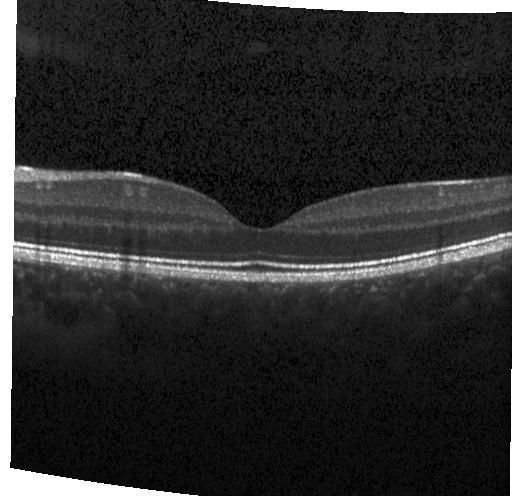

Retinal OCT cross-section · spectral-domain OCT. Finding: no evidence of choroidal neovascularization, diabetic macular edema, or drusen.